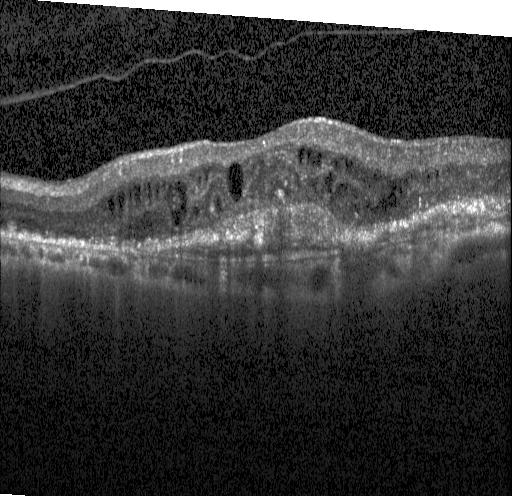
Spectral-domain OCT B-scan: a choroidal neovascular membrane.